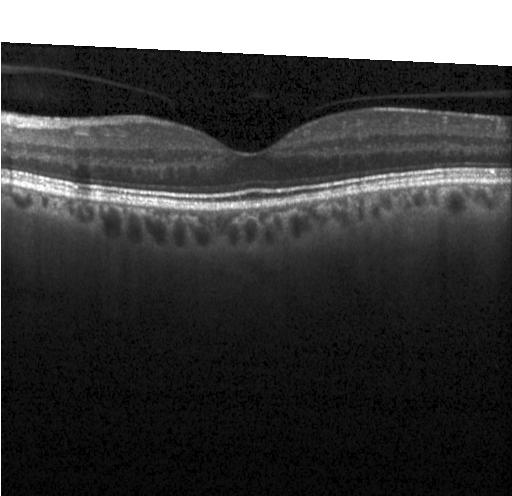
Centered on the fovea · OCT line scan.
Finding: no choroidal neovascularization, diabetic macular edema, or drusen.